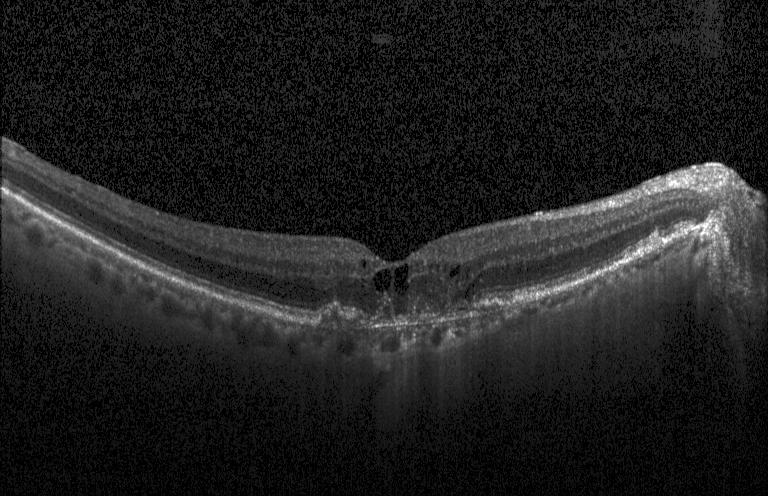 Assessment: a choroidal neovascular membrane.